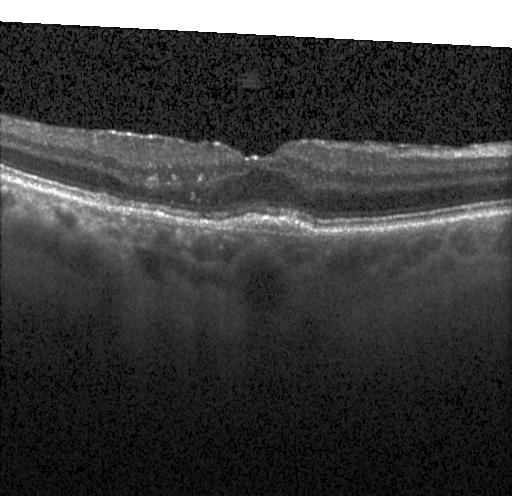 Dx: choroidal neovascularization (CNV).